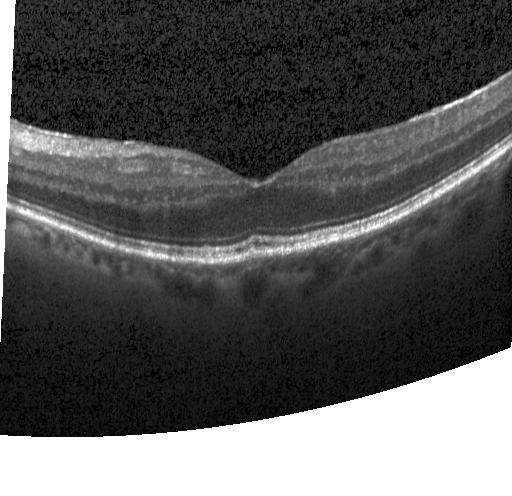
This B-scan demonstrates neither choroidal neovascularization, diabetic macular edema, nor drusen.